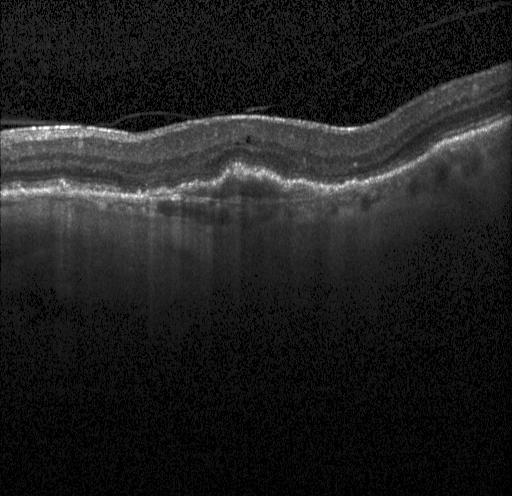

This B-scan demonstrates choroidal neovascularization.